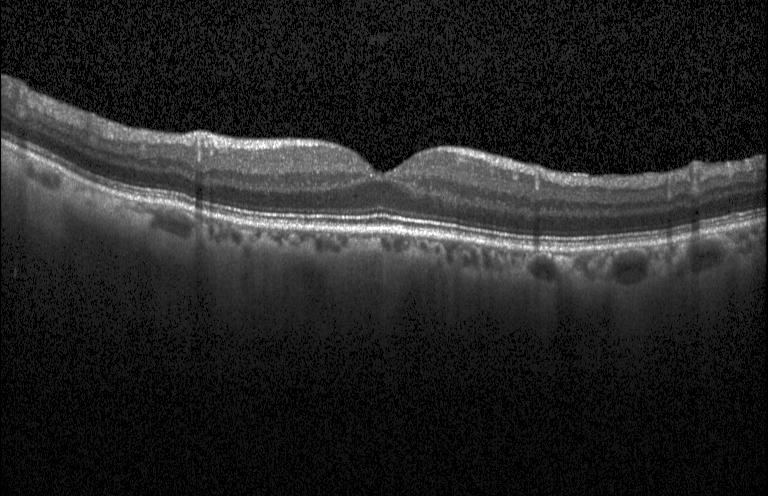
Optical coherence tomography scan, Heidelberg Spectralis OCT system, macular scan
Assessment: neither CNV, DME, nor drusen.